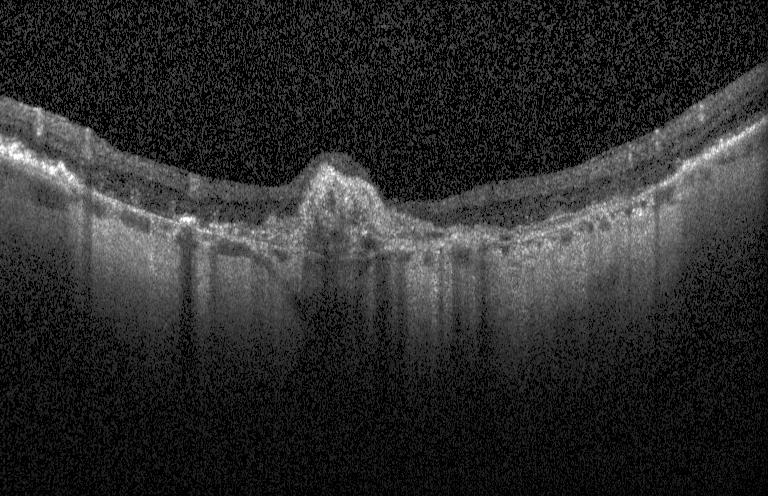
Impression: a choroidal neovascular membrane.